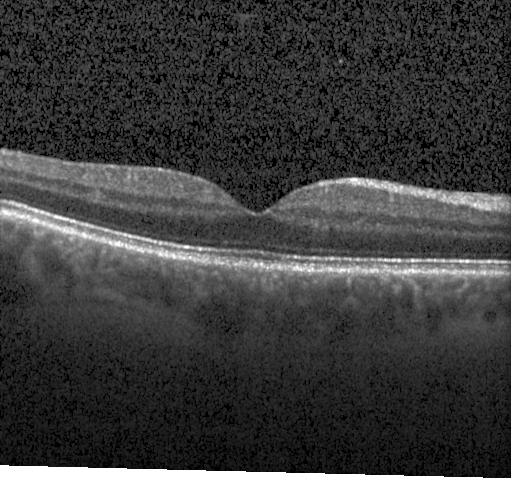

OCT line scan. Diagnosis: no evidence of CNV, DME, or drusen.